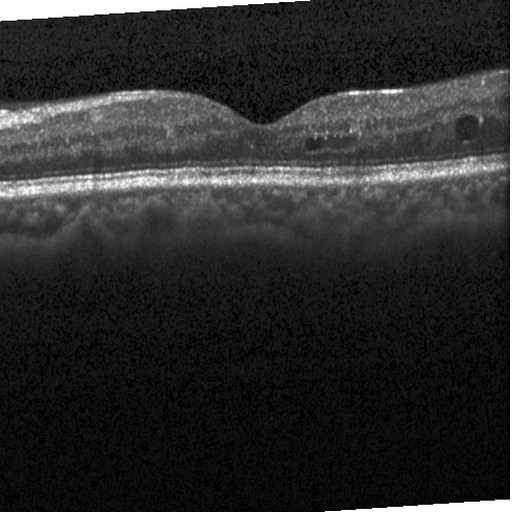
OCT line scan. Impression: DME.